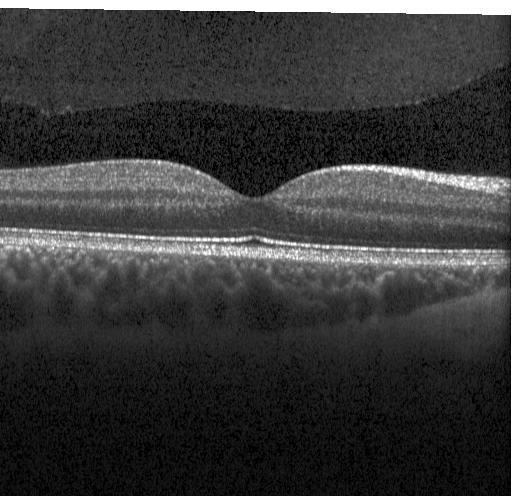
Retinal OCT B-scan. SD-OCT. Through the macula. Instrument: Heidelberg Spectralis. OCT finding: neither CNV, DME, nor drusen.